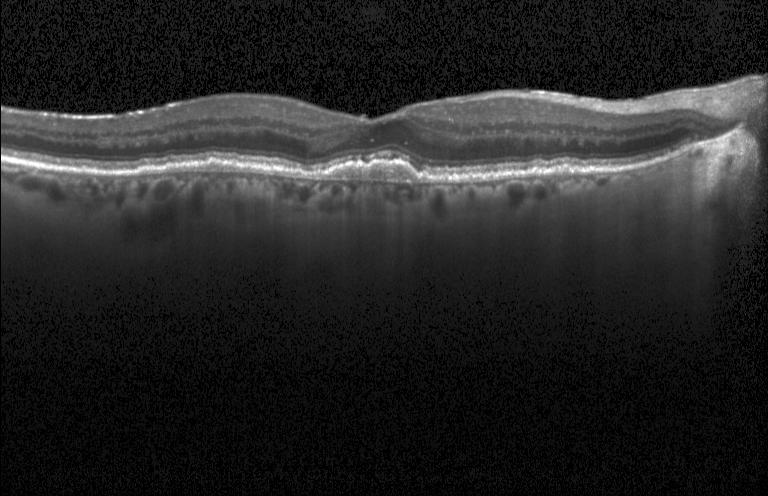
Retinal OCT cross-section — Finding: choroidal neovascularization (CNV).